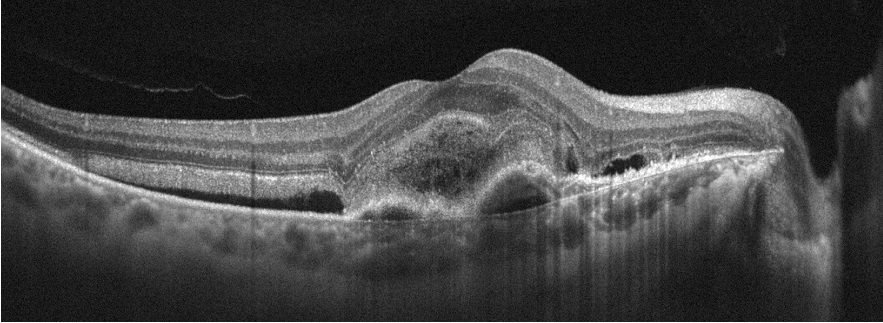
Retinal OCT B-scan
Impression: age-related macular degeneration.